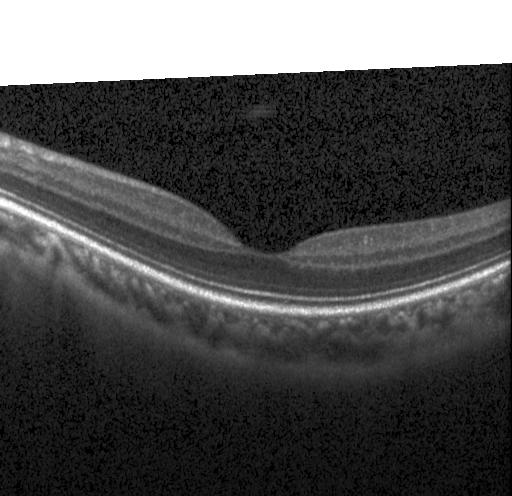

Retinal OCT cross-section showing no choroidal neovascularization, no diabetic macular edema, and no drusen.